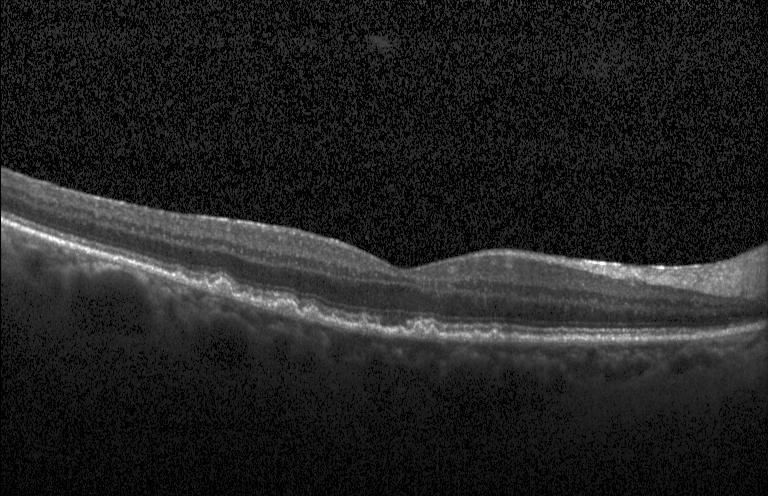 Macular scan; spectral-domain optical coherence tomography; OCT B-scan
Impression: drusen.